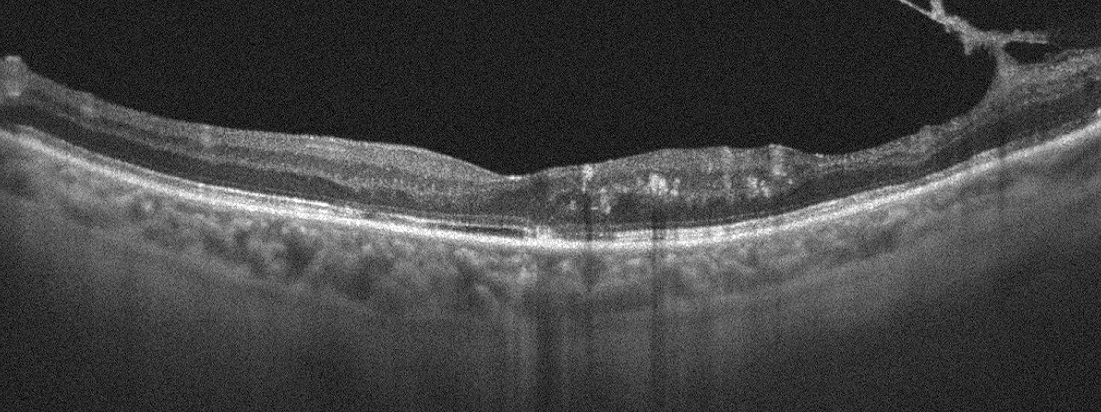

Optical coherence tomography B-scan.
Impression: diabetic macular edema (DME).